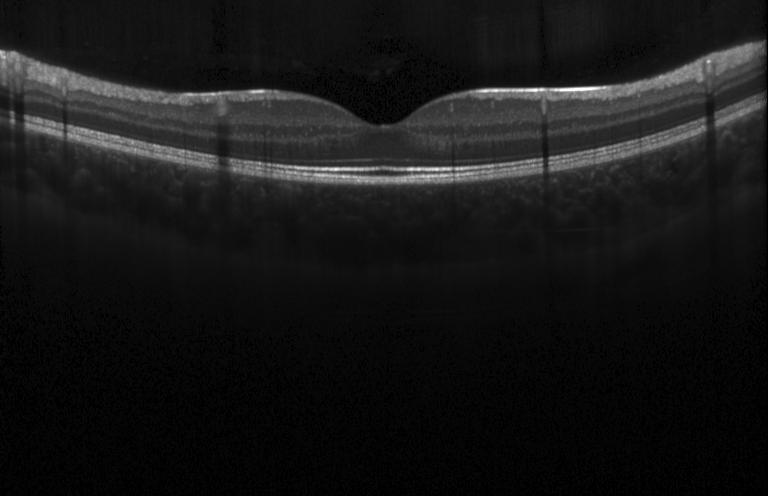 Spectral-domain OCT. OCT line scan.
Assessment: no choroidal neovascularization, no diabetic macular edema, and no drusen.